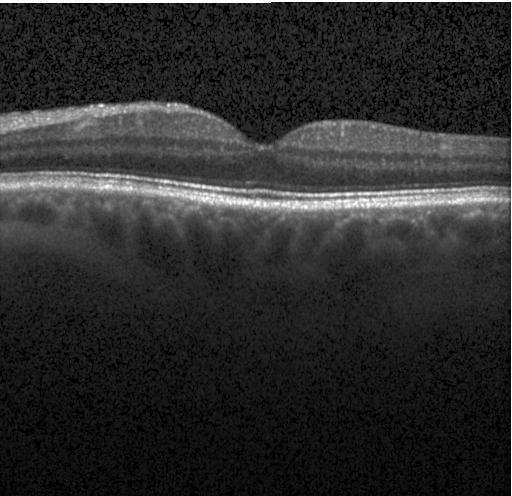

OCT line scan; acquired on a Heidelberg Spectralis — Finding: no choroidal neovascularization, diabetic macular edema, or drusen.